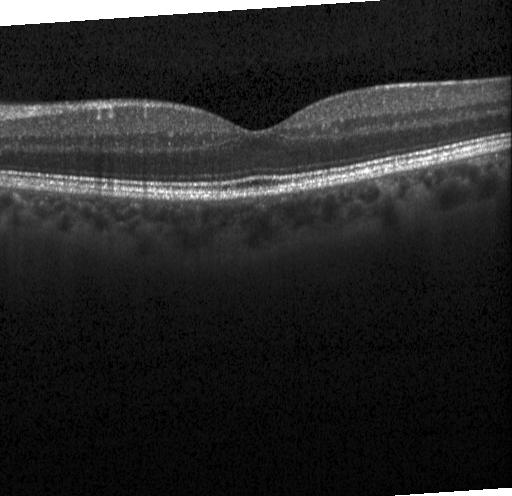 OCT scan showing neither choroidal neovascularization, diabetic macular edema, nor drusen.